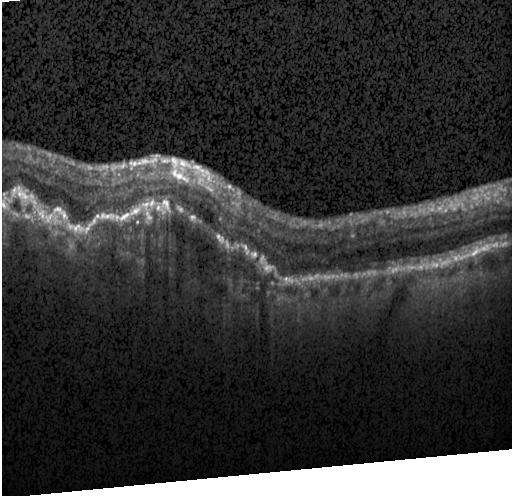 OCT line scan · Heidelberg Spectralis · spectral-domain OCT.
Diagnosis: choroidal neovascularization (CNV).